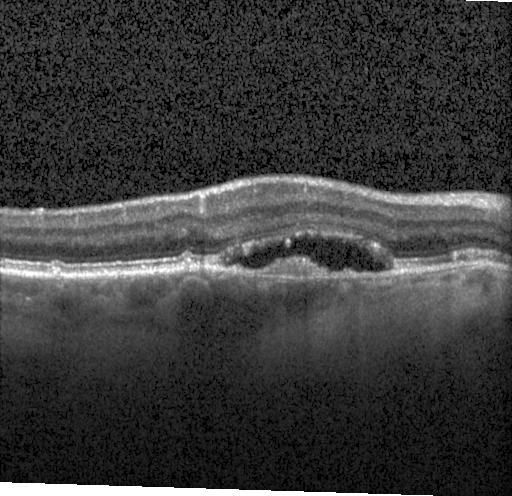
Retinal OCT B-scan — This B-scan demonstrates choroidal neovascularization.